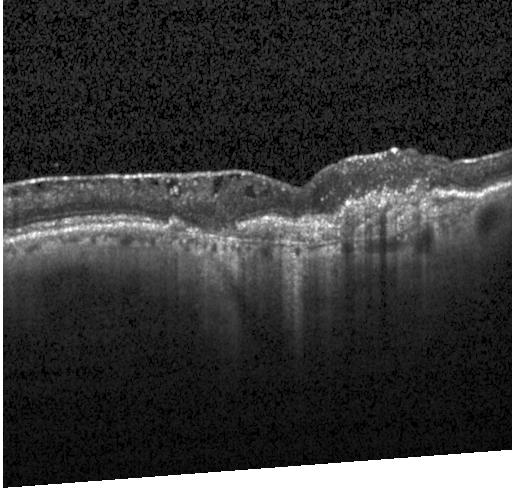
Horizontal scan through the fovea; optical coherence tomography B-scan; spectral-domain OCT.
The scan shows a choroidal neovascular membrane.